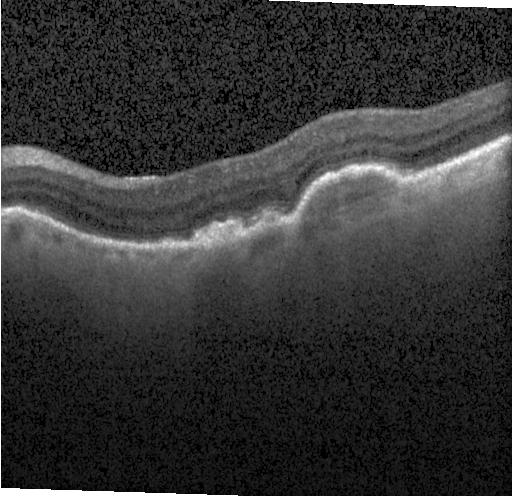 Through the macula, acquired on a Heidelberg Spectralis, spectral-domain OCT, retinal OCT cross-section. Assessment: CNV.